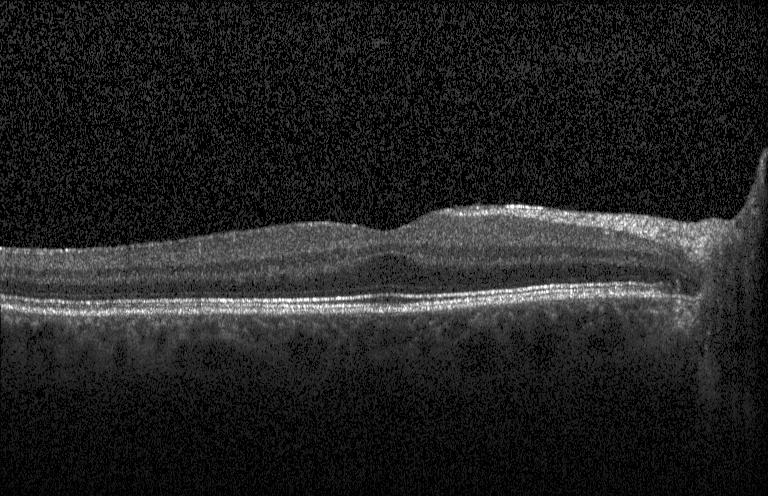

OCT finding: no evidence of choroidal neovascularization, diabetic macular edema, or drusen.